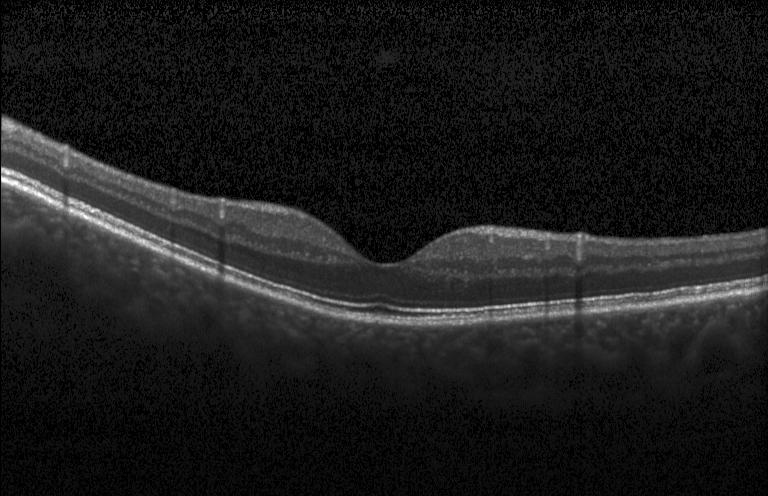 Optical coherence tomography scan
Finding: no choroidal neovascularization, no diabetic macular edema, and no drusen.